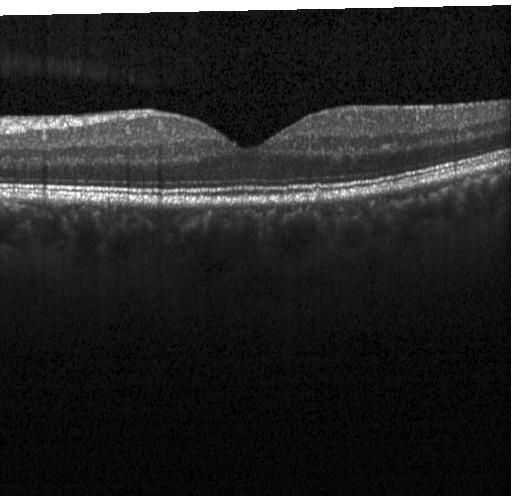
Diagnosis: no CNV, no DME, and no drusen.